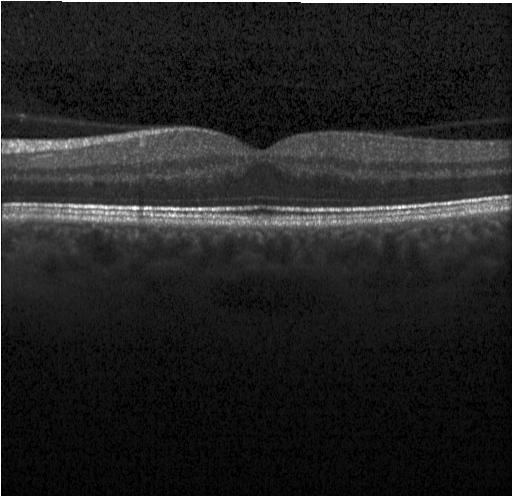 Macular OCT demonstrating no choroidal neovascularization, diabetic macular edema, or drusen.